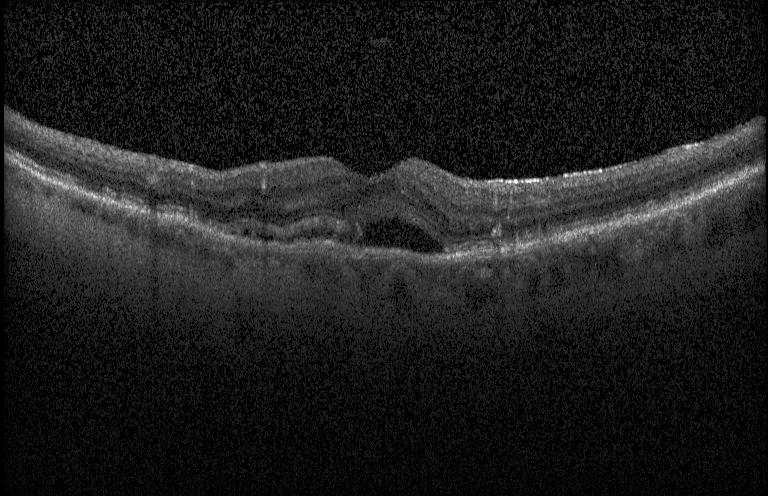 Optical coherence tomography B-scan — CNV.